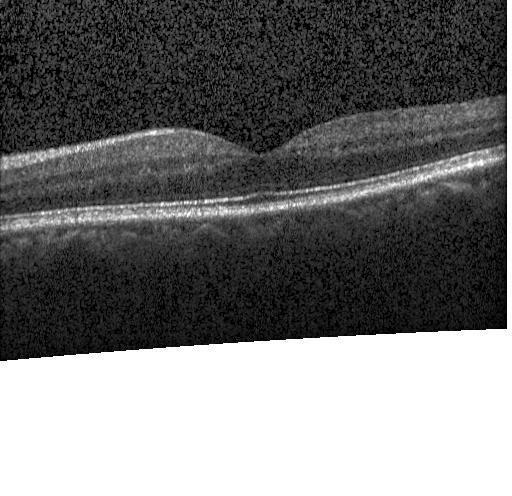
OCT B-scan · SD-OCT · Heidelberg Spectralis. Impression: no choroidal neovascularization, no diabetic macular edema, and no drusen.